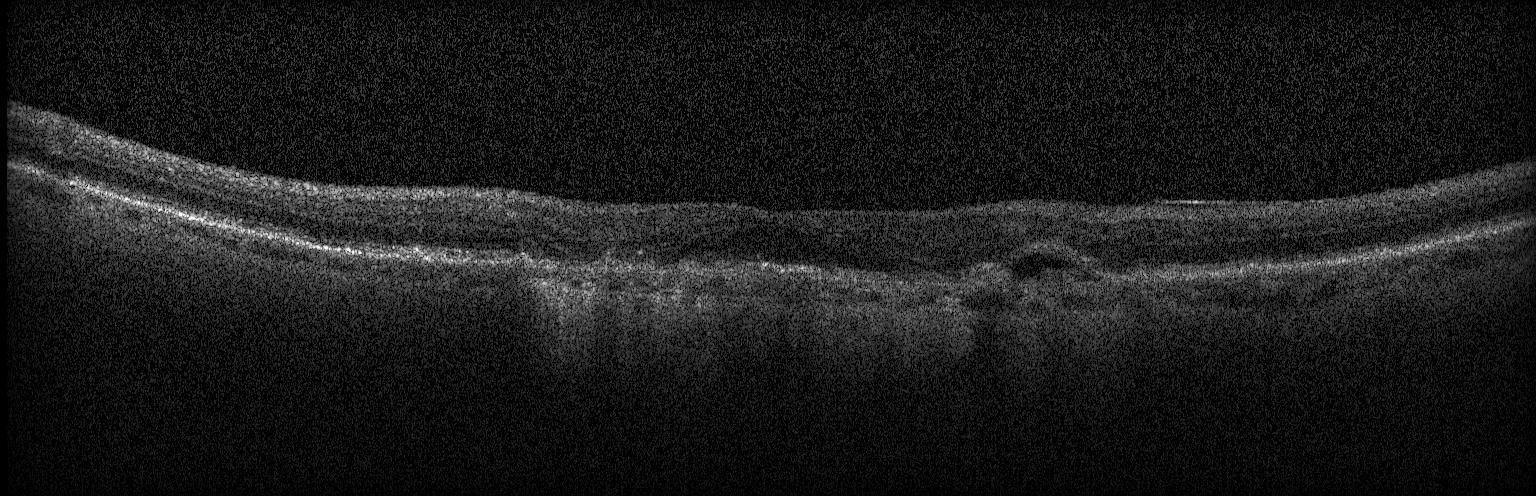
Heidelberg Spectralis OCT system. OCT line scan — Impression: choroidal neovascularization.